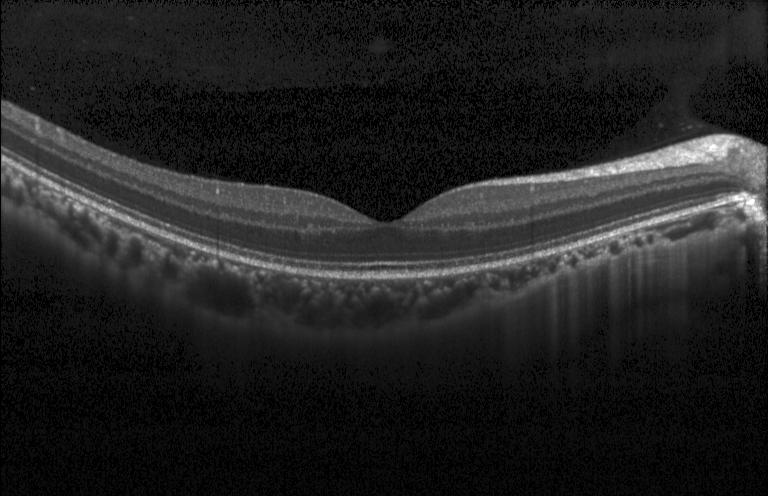
Spectral-domain optical coherence tomography, Heidelberg Spectralis, retinal OCT cross-section, macular scan. Impression: neither CNV, DME, nor drusen.